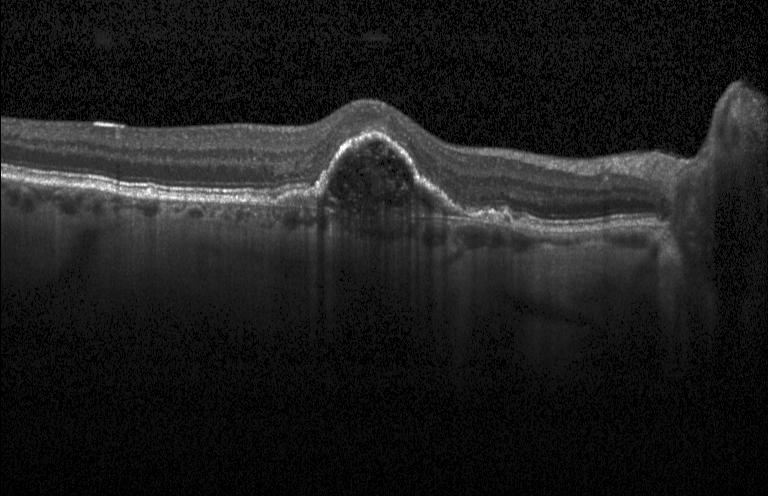
Fovea-centered. Spectral-domain OCT. Heidelberg Spectralis. Optical coherence tomography B-scan
Macular OCT: choroidal neovascularization.